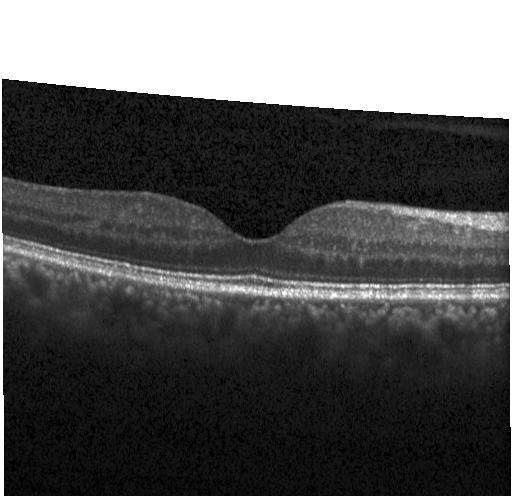

Impression: no choroidal neovascularization, no diabetic macular edema, and no drusen.